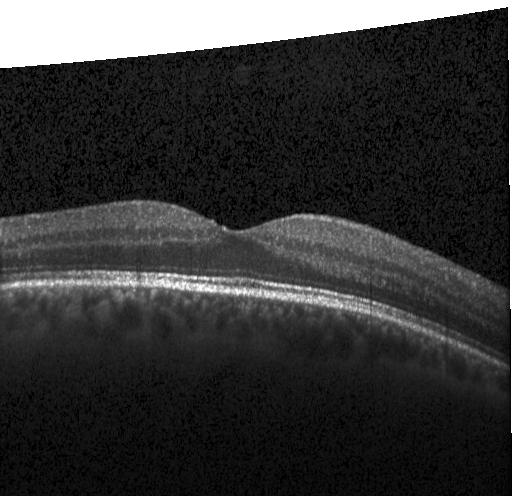

Spectral-domain optical coherence tomography; optical coherence tomography scan
OCT finding: no choroidal neovascularization, diabetic macular edema, or drusen.